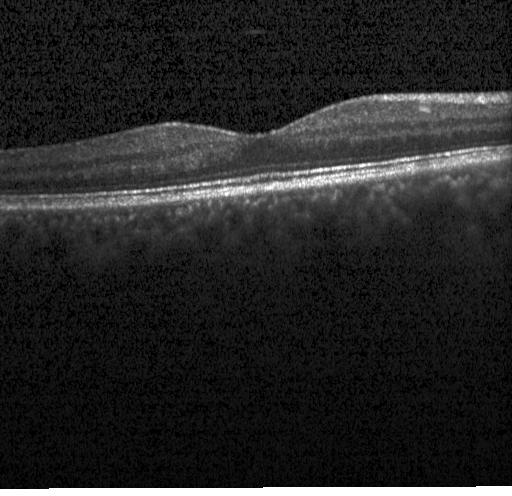

The scan shows no choroidal neovascularization, no diabetic macular edema, and no drusen.